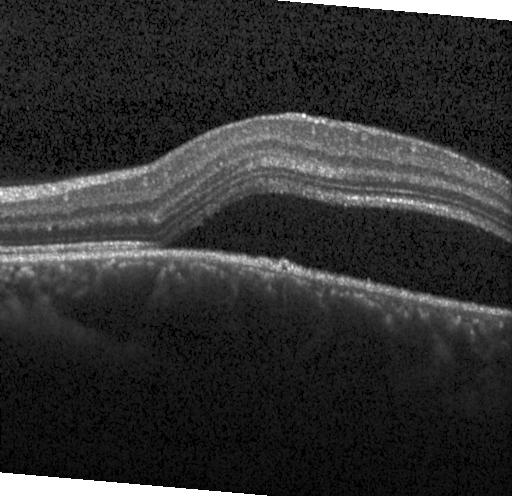 Retinal OCT cross-section. Spectral-domain OCT. Assessment: a choroidal neovascular membrane.